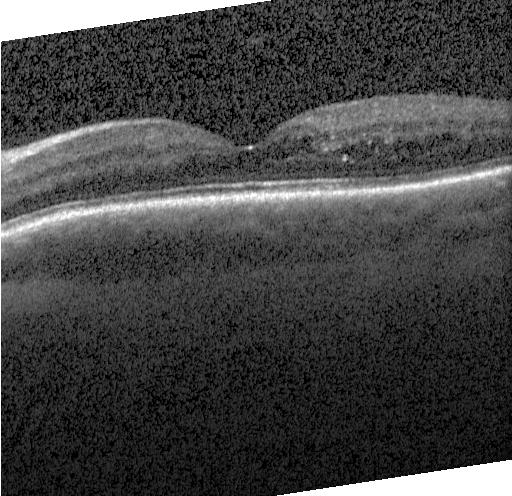 Centered on the fovea; optical coherence tomography B-scan; spectral-domain OCT; Heidelberg Spectralis OCT system
The scan shows diabetic macular edema.